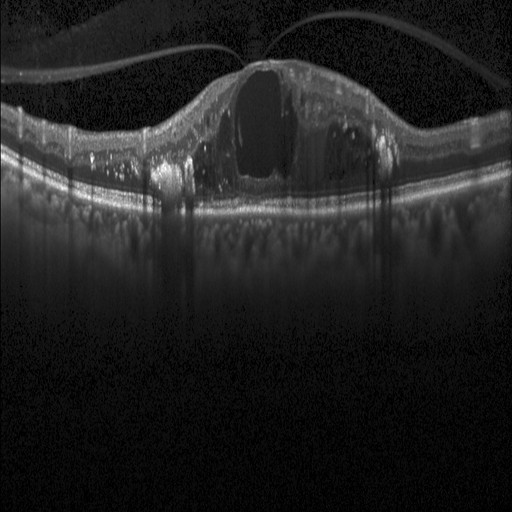

Diagnosis: DME.